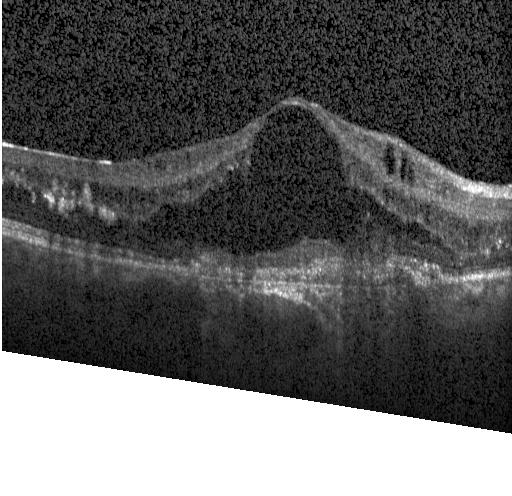
Optical coherence tomography B-scan
Choroidal neovascularization (CNV).